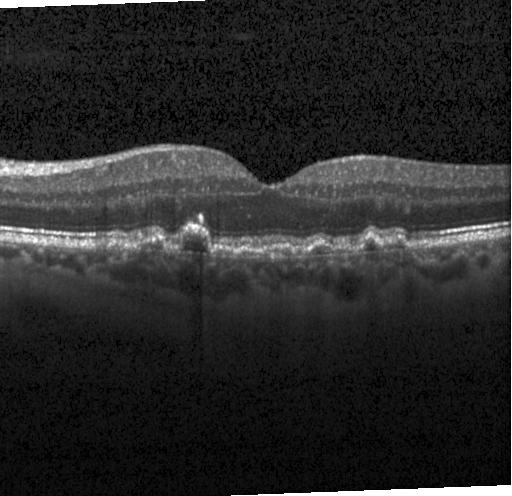
SD-OCT; OCT B-scan; centered on the fovea
Diagnosis: drusen.